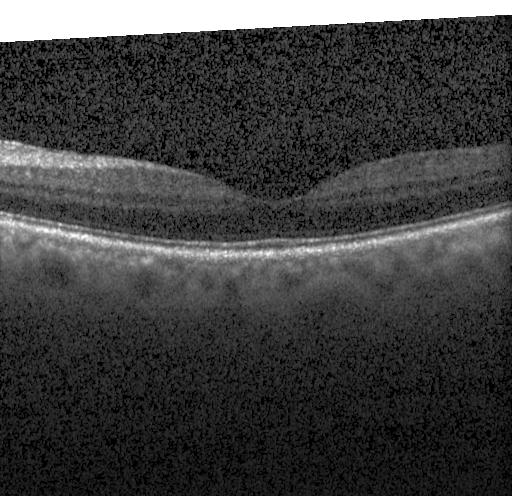
Diagnosis: no CNV, DME, or drusen.